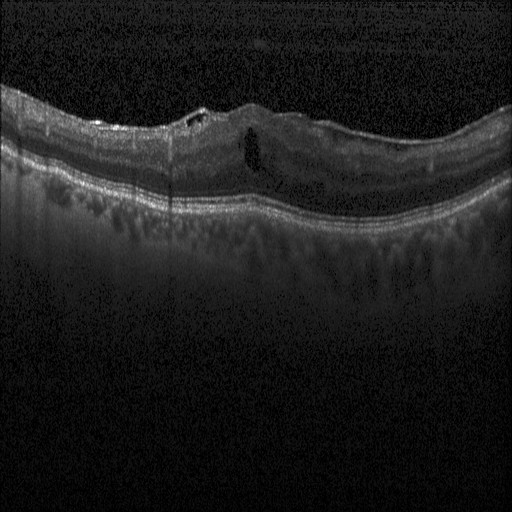

Optical coherence tomography B-scan. SD-OCT. Horizontal scan through the fovea. Heidelberg Spectralis.
Diabetic macular edema (DME).